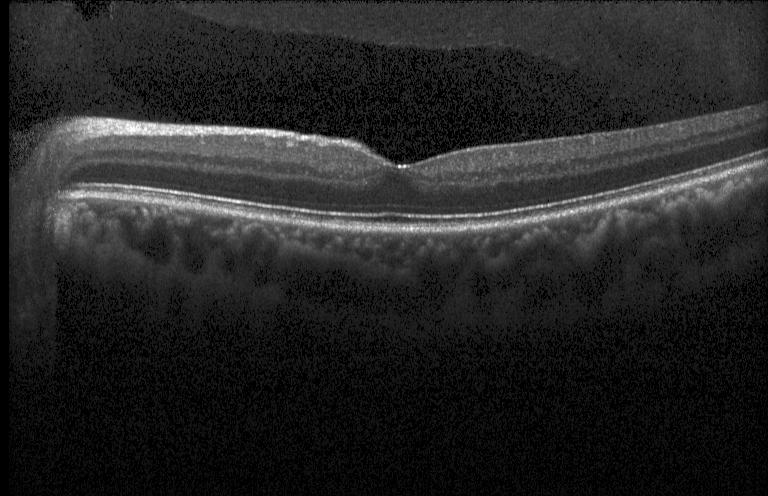 Instrument: Heidelberg Spectralis; spectral-domain optical coherence tomography; optical coherence tomography scan; horizontal scan through the fovea
OCT finding: neither choroidal neovascularization, diabetic macular edema, nor drusen.